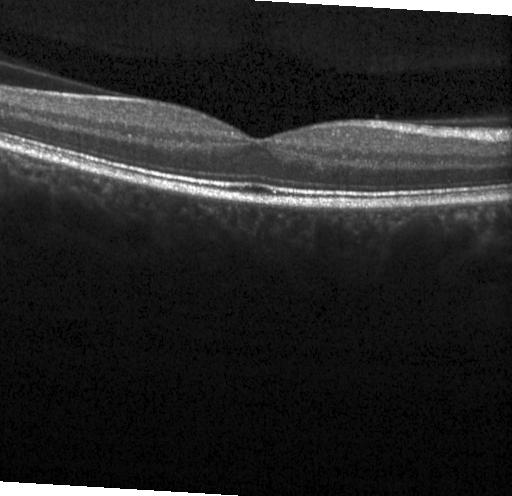

This B-scan demonstrates neither choroidal neovascularization, diabetic macular edema, nor drusen.